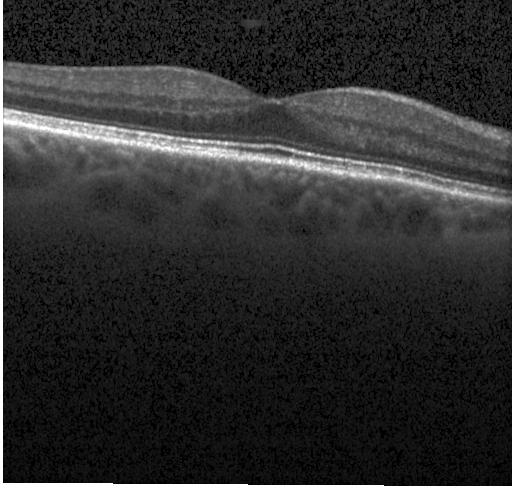
OCT scan showing no choroidal neovascularization, no diabetic macular edema, and no drusen.